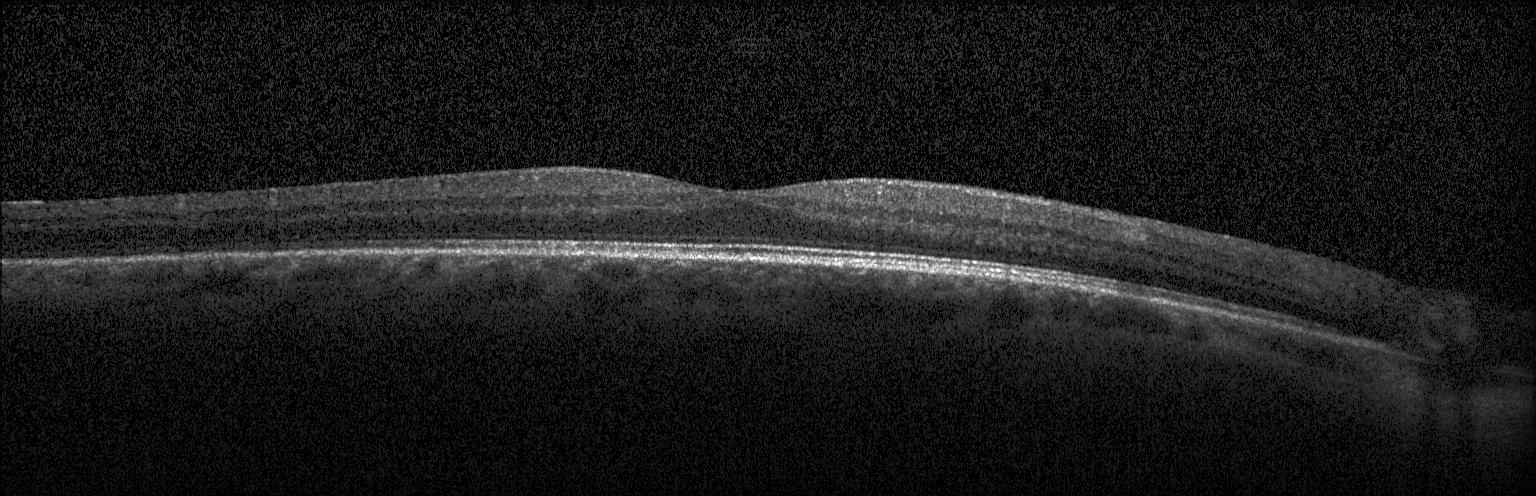
Retinal OCT cross-section.
Diagnosis: no evidence of CNV, DME, or drusen.